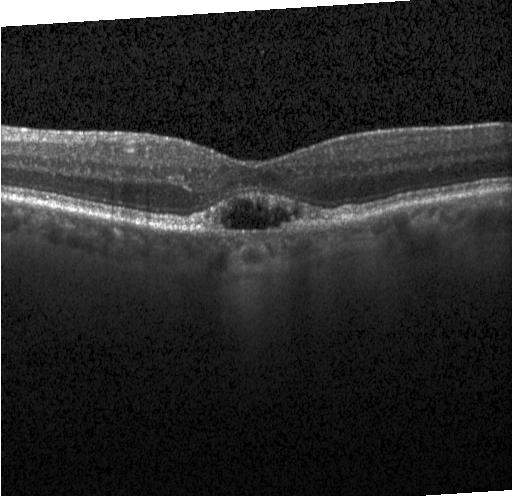
Spectral-domain optical coherence tomography; macular scan; OCT line scan; Heidelberg Spectralis
Choroidal neovascularization.